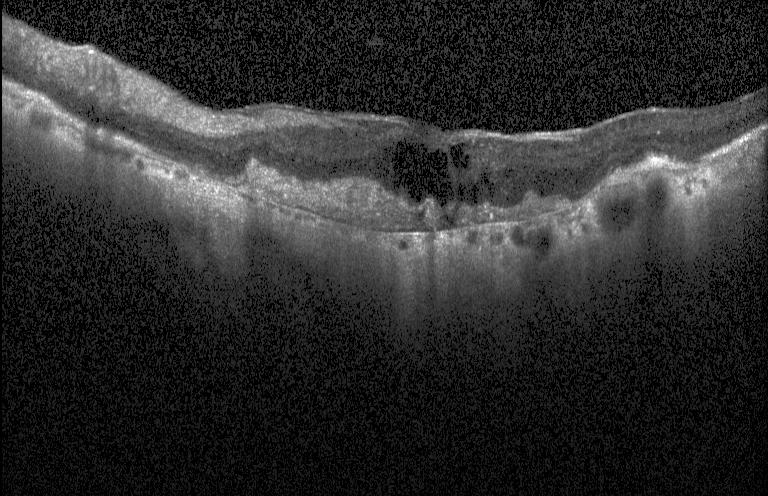

OCT line scan. Spectral-domain optical coherence tomography. Fovea-centered. Instrument: Heidelberg Spectralis.
Dx: a choroidal neovascular membrane.